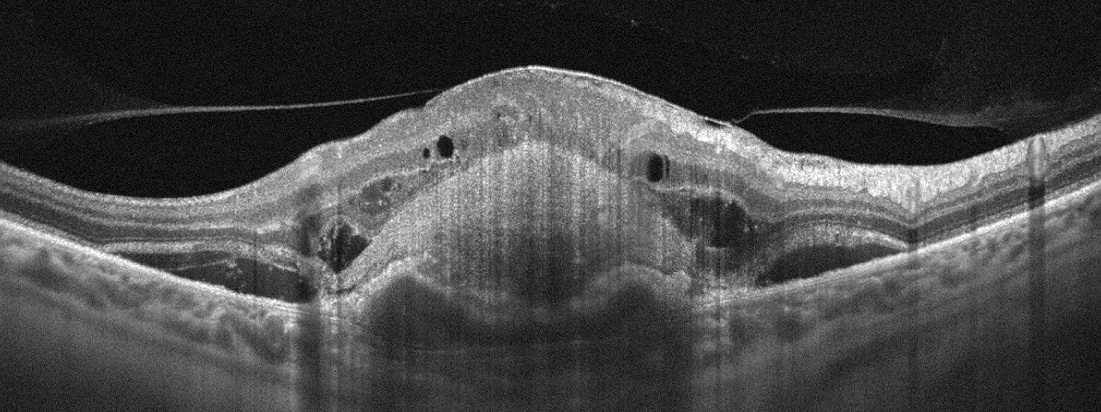 OCT B-scan. Instrument: Optovue Avanti RTVue XR. Finding: age-related macular degeneration.